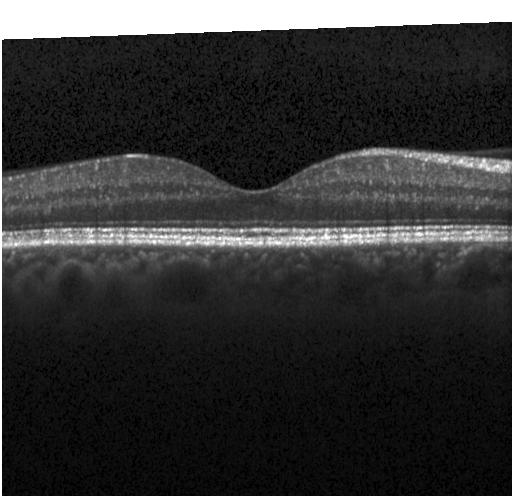 OCT finding: no evidence of choroidal neovascularization, diabetic macular edema, or drusen.